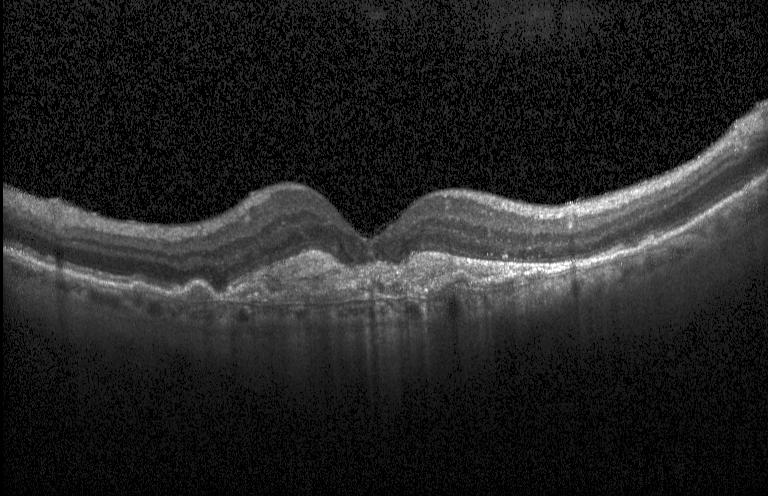

Optical coherence tomography B-scan
Impression: CNV.